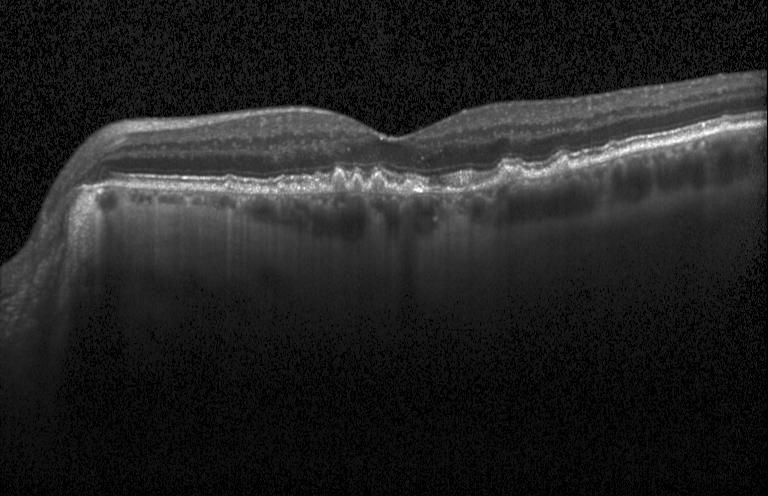
OCT B-scan showing sub-RPE drusenoid deposits.